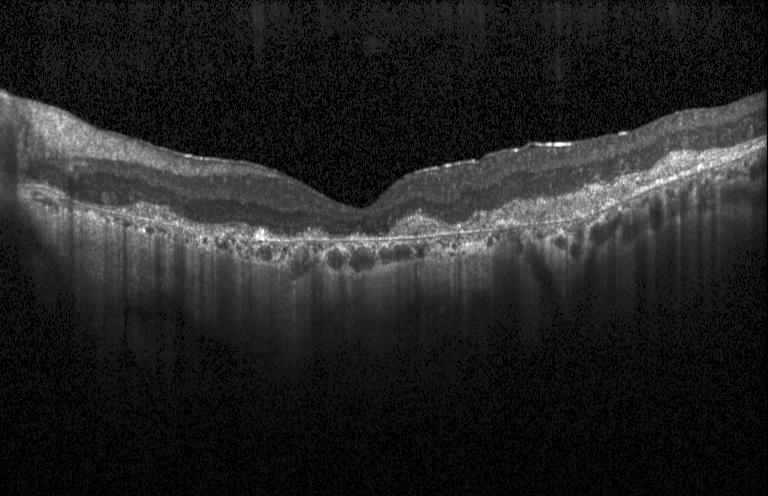 Optical coherence tomography scan. Heidelberg Spectralis. Spectral-domain optical coherence tomography. Macular scan.
Impression: a choroidal neovascular membrane.